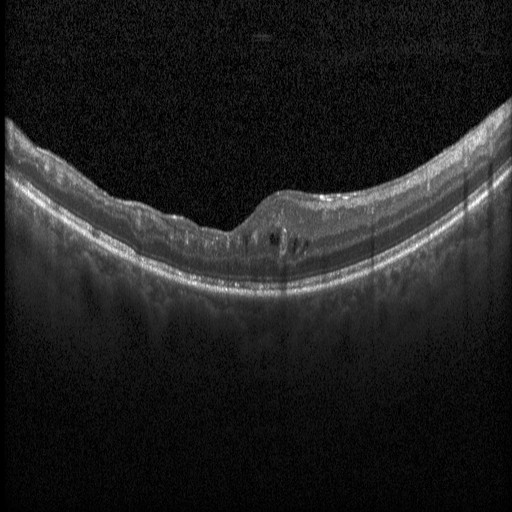

Macular scan · instrument: Heidelberg Spectralis · optical coherence tomography scan. Finding: diabetic macular edema.